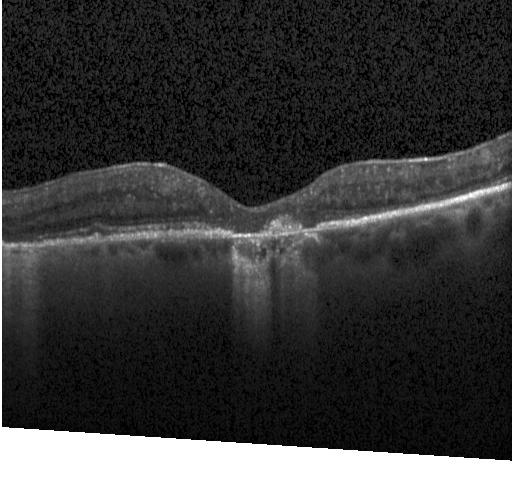
OCT B-scan; spectral-domain optical coherence tomography; centered on the fovea; Heidelberg Spectralis OCT system
CNV.